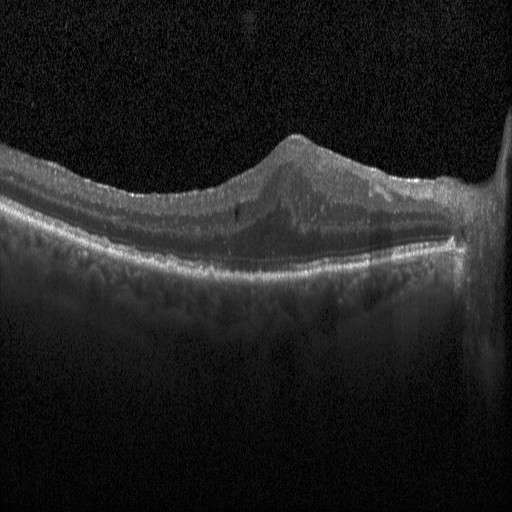
This B-scan demonstrates diabetic macular edema (DME).